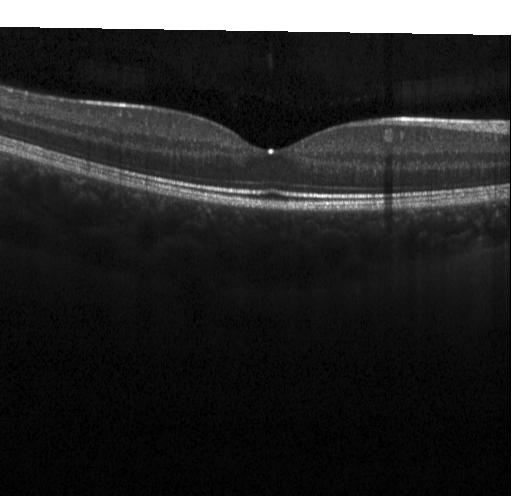 OCT line scan. Assessment: neither CNV, DME, nor drusen.